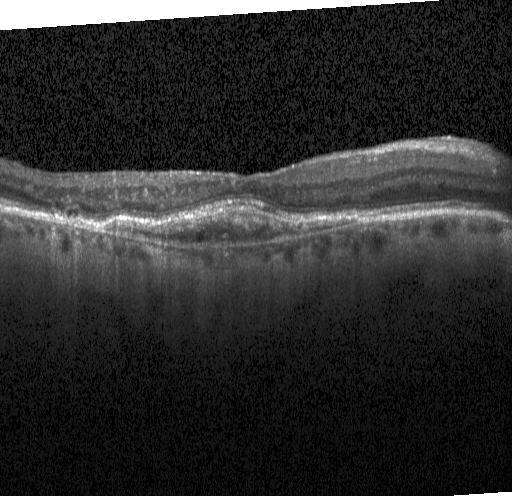 Retinal OCT cross-section.
Diagnosis: choroidal neovascularization.